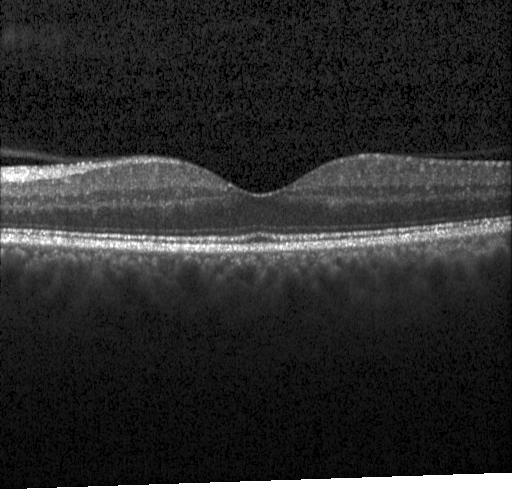 SD-OCT, macular scan, acquired on a Heidelberg Spectralis, OCT B-scan
OCT finding: no evidence of CNV, DME, or drusen.